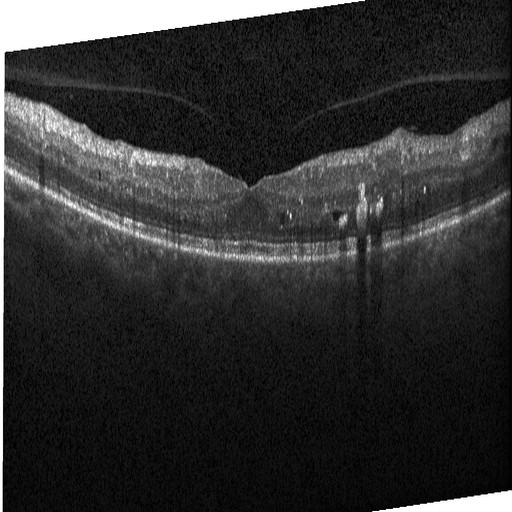
Retinal OCT cross-section, spectral-domain OCT, Heidelberg Spectralis
Finding: diabetic macular edema.